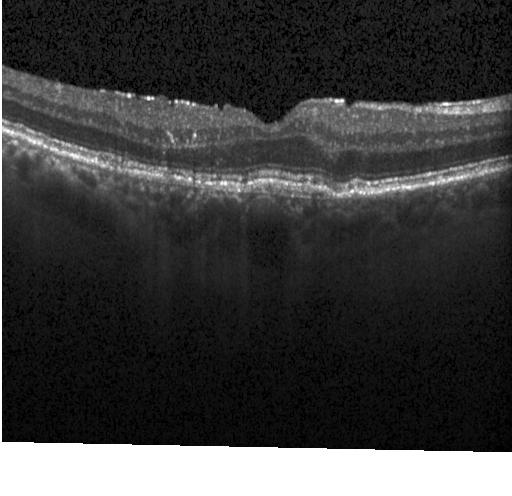 Spectral-domain optical coherence tomography, retinal OCT B-scan.
OCT finding: choroidal neovascularization.